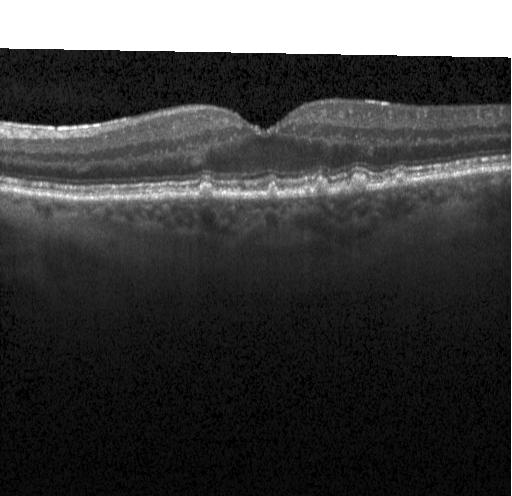 Diagnosis: multiple drusen.